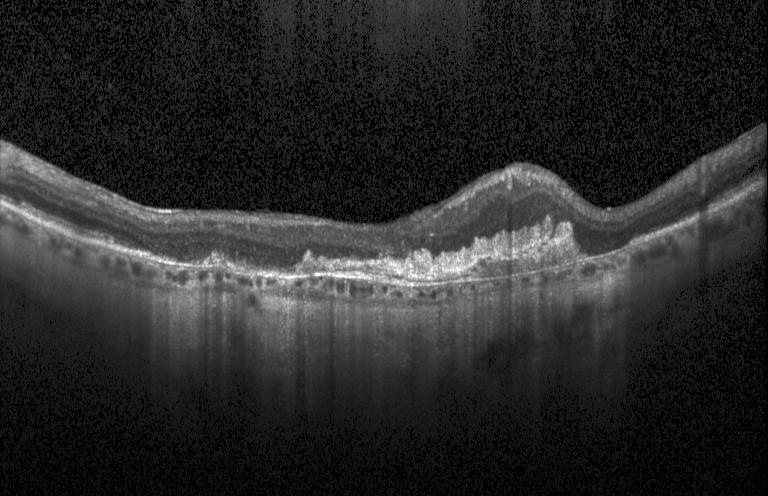
Instrument: Heidelberg Spectralis · retinal OCT B-scan.
Assessment: CNV.